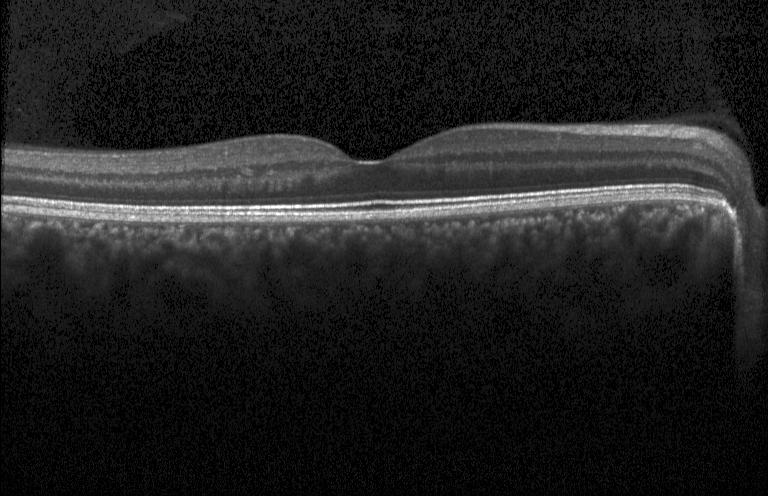 Retinal OCT cross-section, instrument: Heidelberg Spectralis, SD-OCT, fovea-centered.
Diagnosis: no evidence of CNV, DME, or drusen.